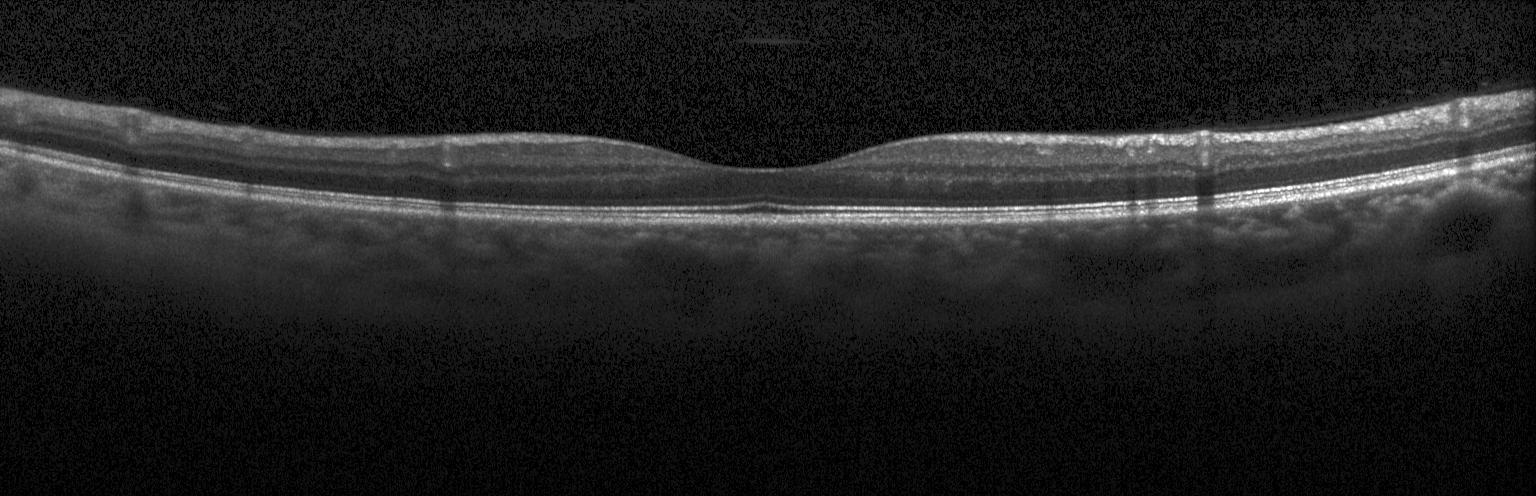 Optical coherence tomography scan · Heidelberg Spectralis OCT system · spectral-domain optical coherence tomography. Finding: no choroidal neovascularization, diabetic macular edema, or drusen.